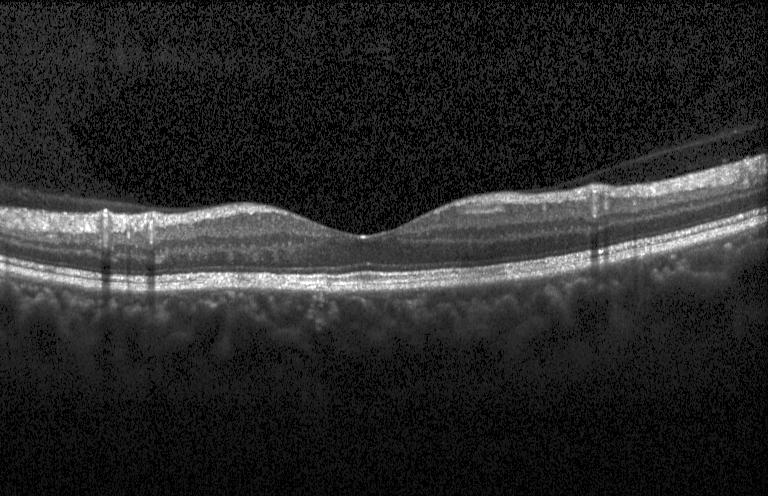
Optical coherence tomography scan; Heidelberg Spectralis OCT system; macular scan; SD-OCT.
Macular OCT: no evidence of CNV, DME, or drusen.